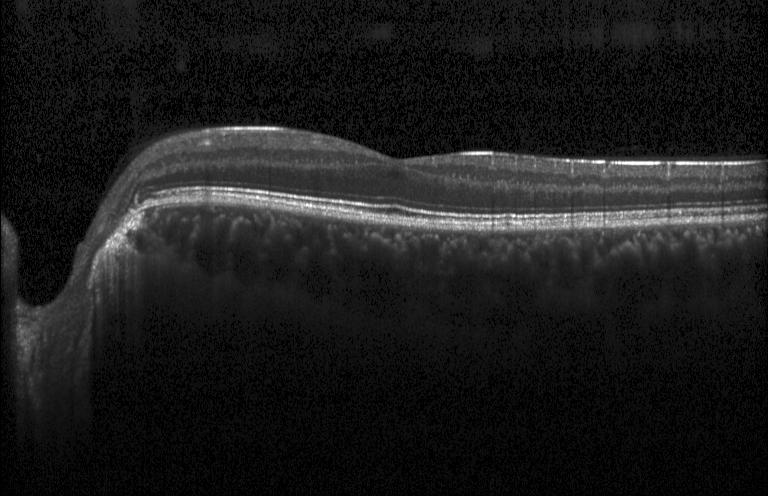

Retinal OCT B-scan · centered on the fovea · Heidelberg Spectralis OCT system · SD-OCT
This B-scan demonstrates no choroidal neovascularization, no diabetic macular edema, and no drusen.